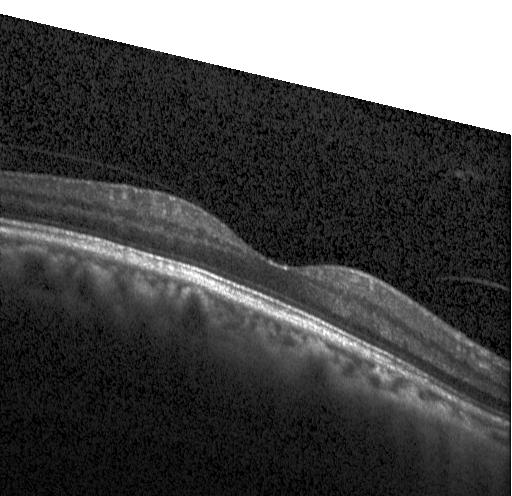 OCT B-scan — Diagnosis: no CNV, no DME, and no drusen.